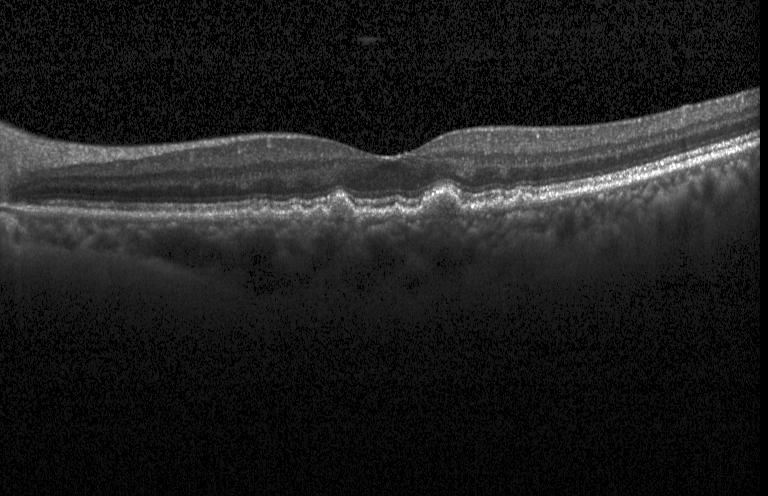

Assessment: drusen.